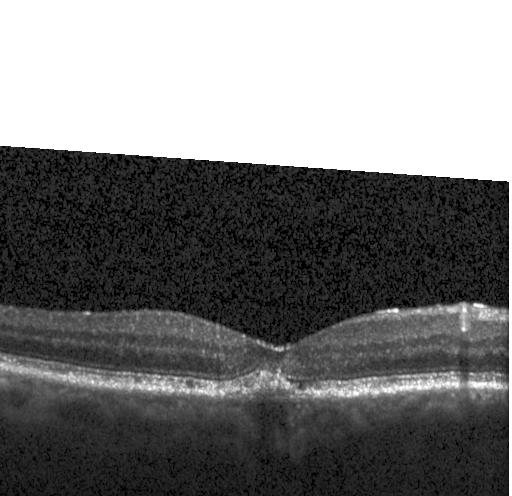
Impression: multiple drusen.